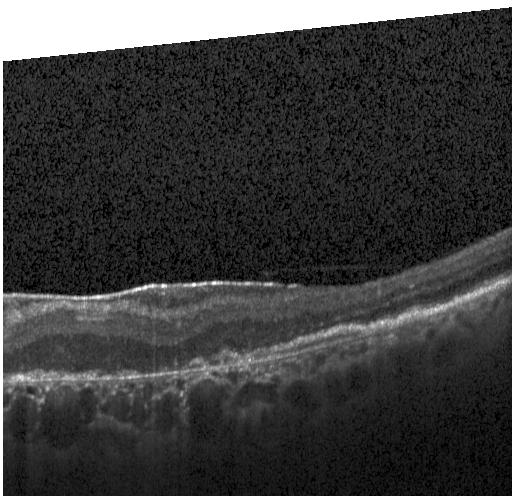

Retinal OCT cross-section; through the macula; Heidelberg Spectralis OCT system; SD-OCT
Impression: a choroidal neovascular membrane.